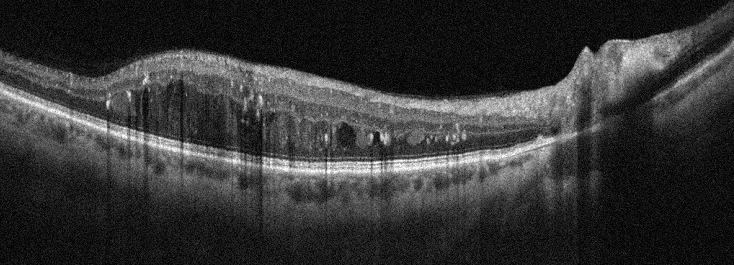

Diagnosis: DME.